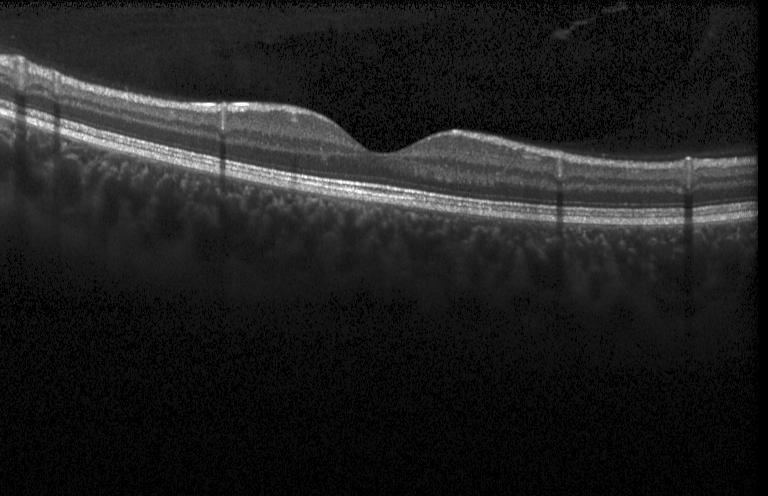

Optical coherence tomography scan. Dx: no choroidal neovascularization, diabetic macular edema, or drusen.